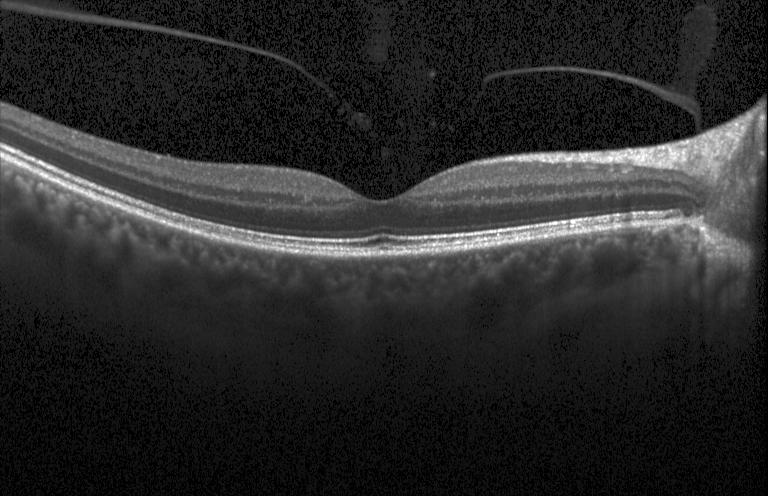
Retinal OCT cross-section showing no choroidal neovascularization, no diabetic macular edema, and no drusen.